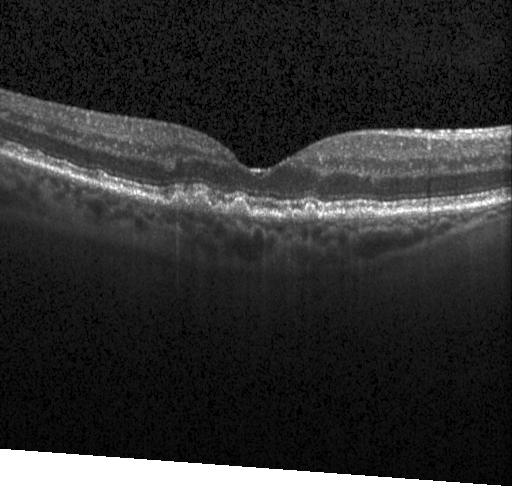

Finding: sub-RPE drusenoid deposits.